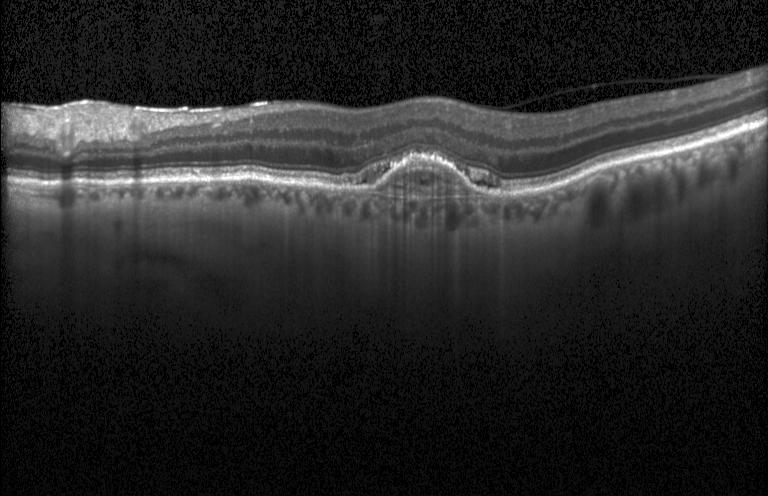
Optical coherence tomography scan — Dx: CNV.